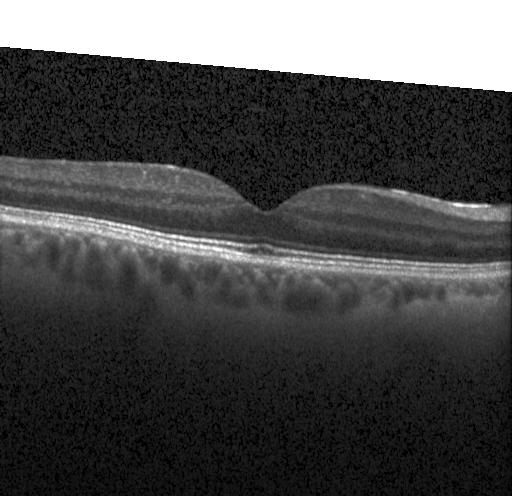
OCT scan showing neither choroidal neovascularization, diabetic macular edema, nor drusen.